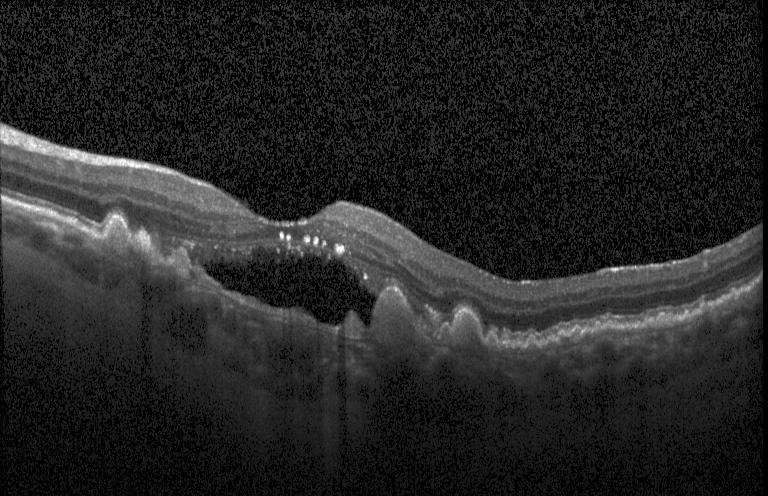
OCT scan showing choroidal neovascularization (CNV).